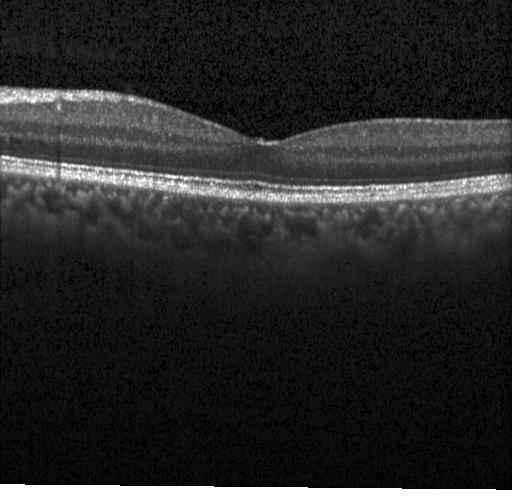

Spectral-domain OCT; macular scan; instrument: Heidelberg Spectralis; OCT line scan. Finding: no choroidal neovascularization, no diabetic macular edema, and no drusen.